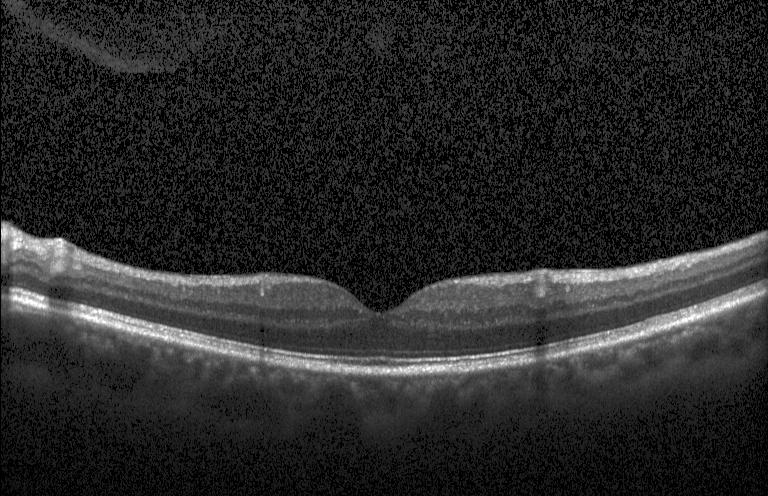

Instrument: Heidelberg Spectralis. Retinal OCT B-scan. Spectral-domain optical coherence tomography
The scan shows no evidence of CNV, DME, or drusen.